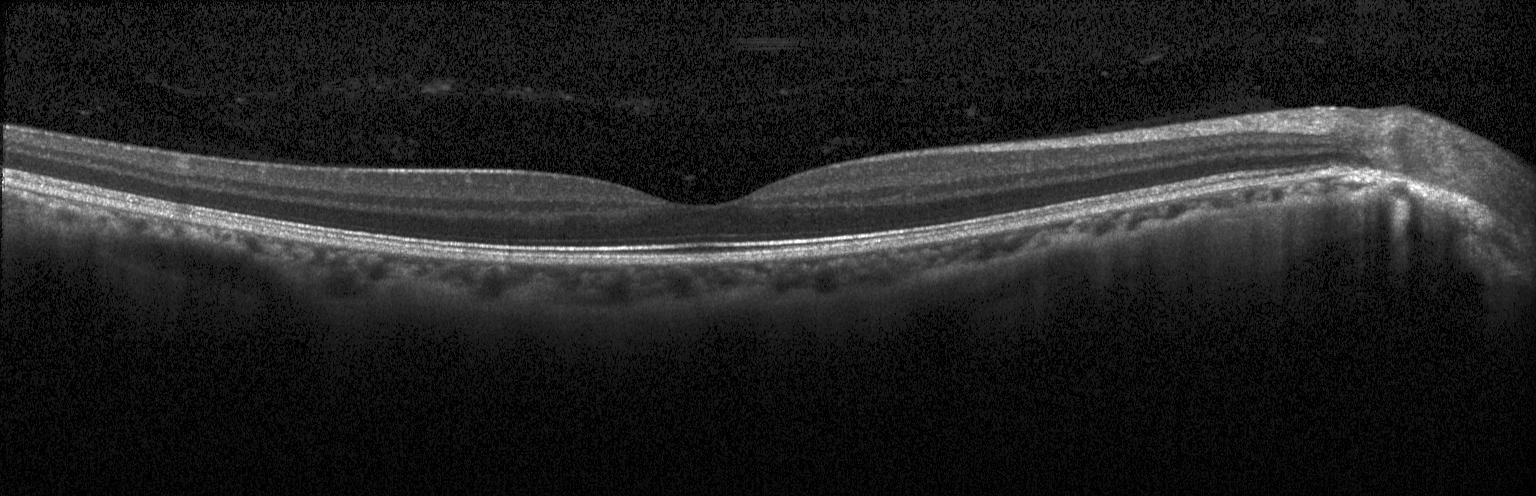
Macular OCT: no evidence of choroidal neovascularization, diabetic macular edema, or drusen.